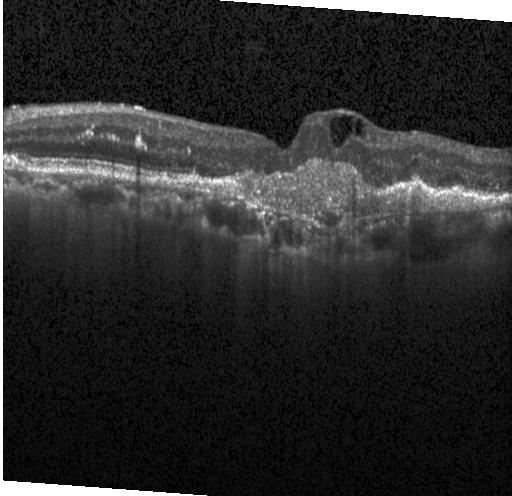

Finding: a choroidal neovascular membrane.